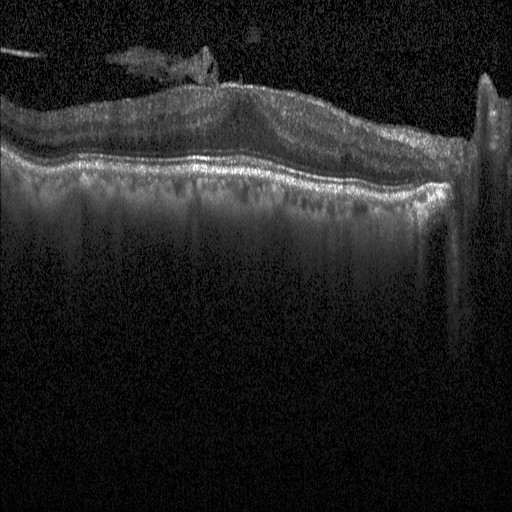 Impression: diabetic macular edema.